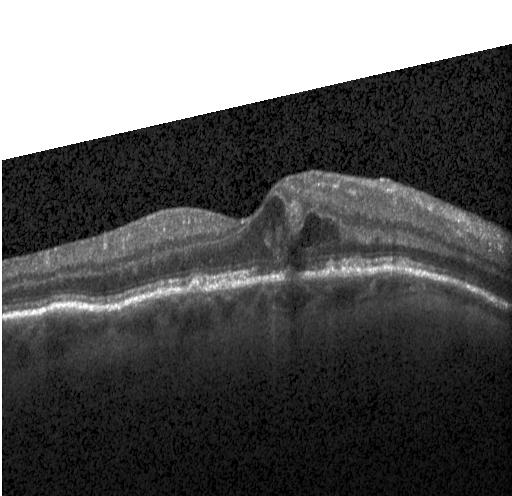
Optical coherence tomography B-scan; spectral-domain optical coherence tomography. The scan shows choroidal neovascularization (CNV).